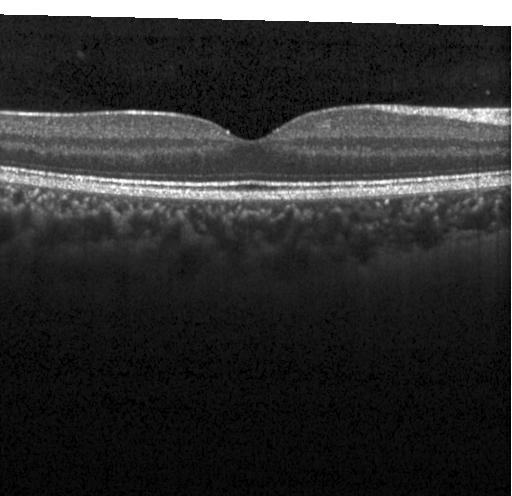
Retinal OCT cross-section · through the macula. Macular OCT: no evidence of choroidal neovascularization, diabetic macular edema, or drusen.